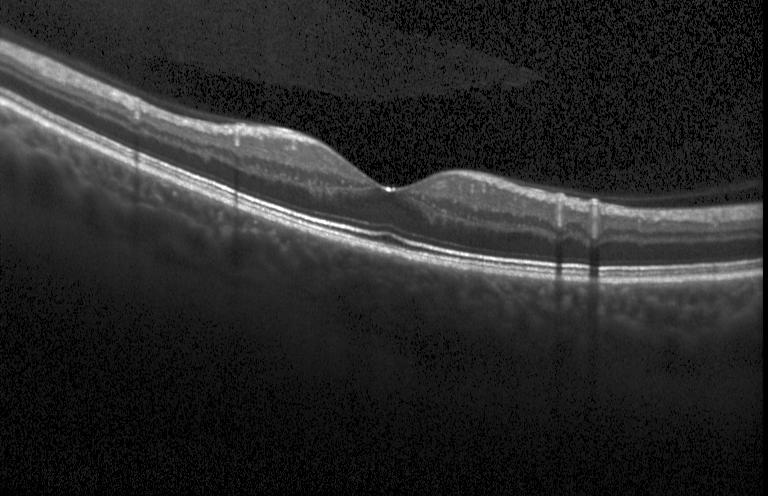

No choroidal neovascularization, no diabetic macular edema, and no drusen.